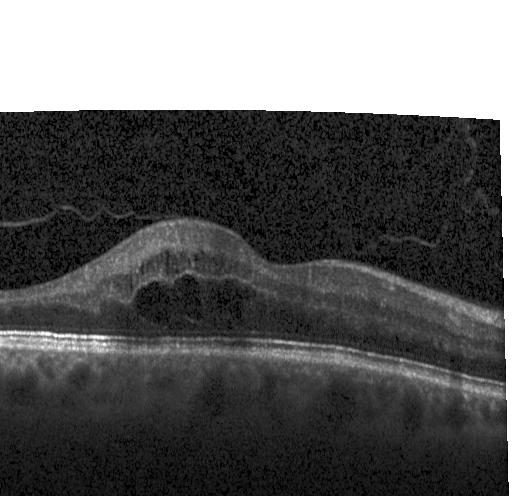 Acquired on a Heidelberg Spectralis, retinal OCT cross-section, spectral-domain optical coherence tomography — Diagnosis: DME.